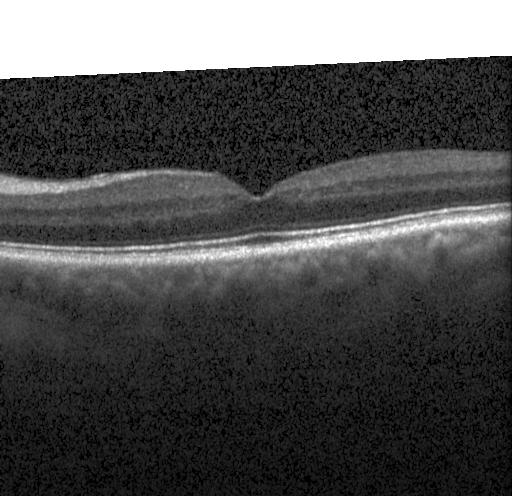 Spectral-domain OCT B-scan: no CNV, no DME, and no drusen.